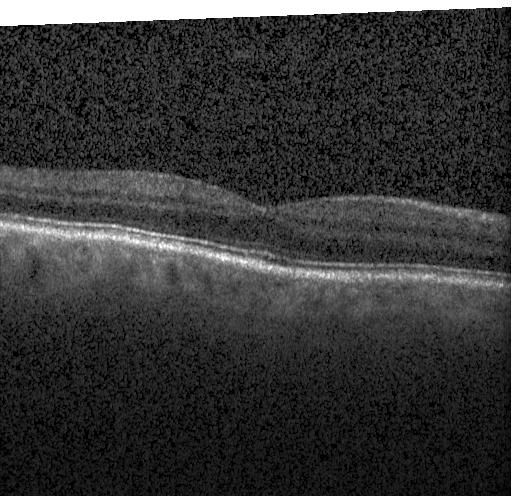
Optical coherence tomography scan, SD-OCT.
Impression: no CNV, DME, or drusen.